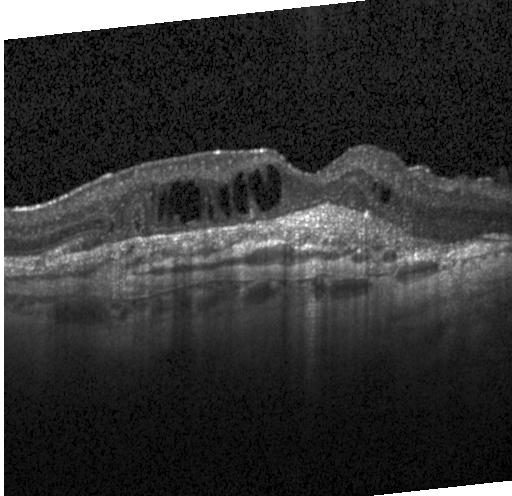 OCT finding: choroidal neovascularization (CNV).